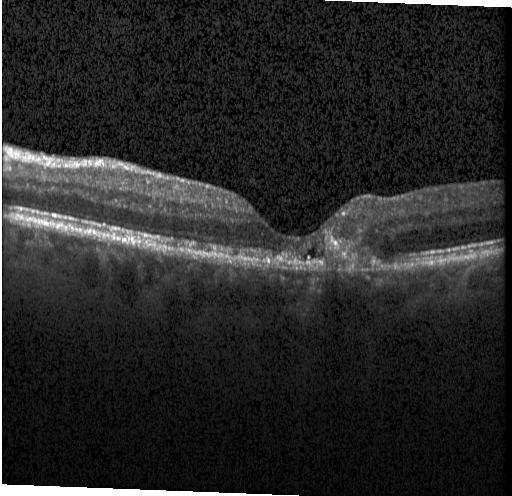 Diagnosis: choroidal neovascularization.